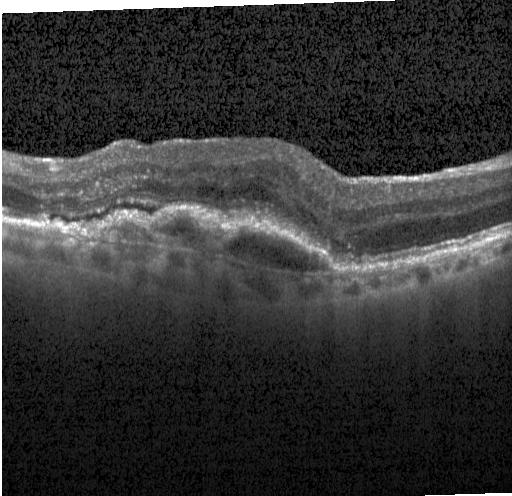 Optical coherence tomography scan — Dx: a choroidal neovascular membrane.